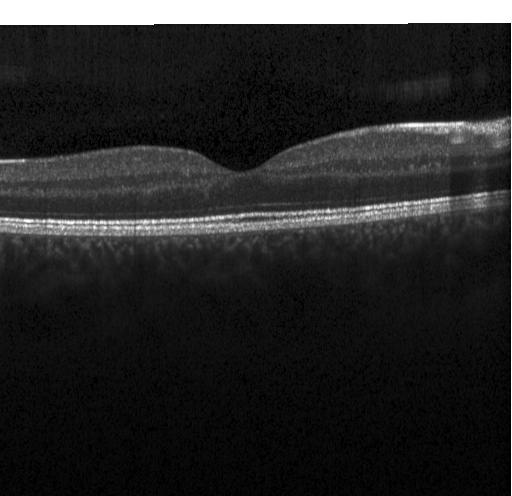

Macular scan. OCT line scan. Spectral-domain OCT
Macular OCT: neither CNV, DME, nor drusen.